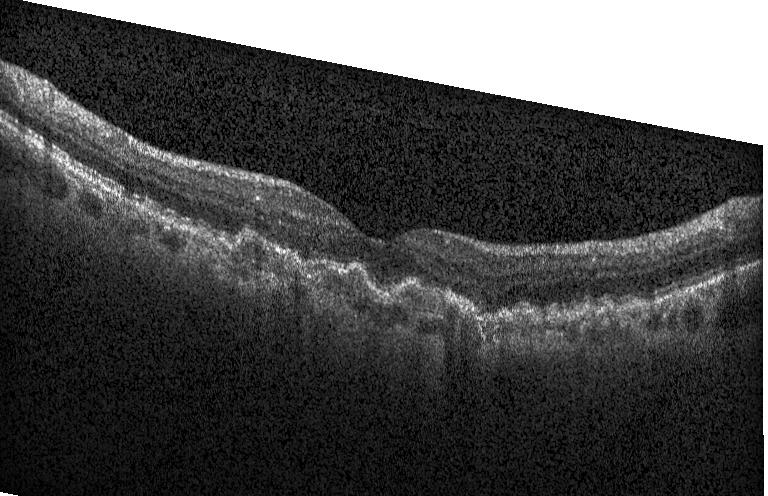
A choroidal neovascular membrane.